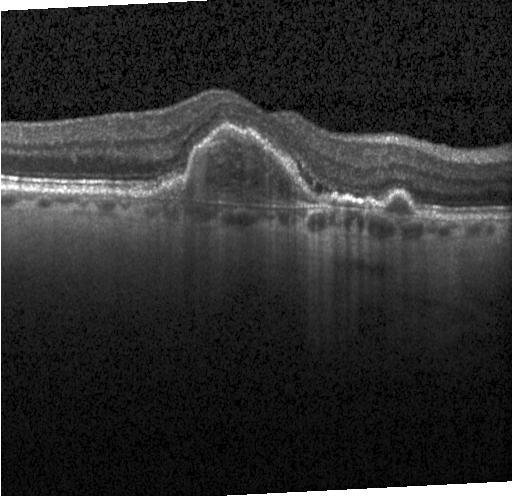

Diagnosis: CNV.